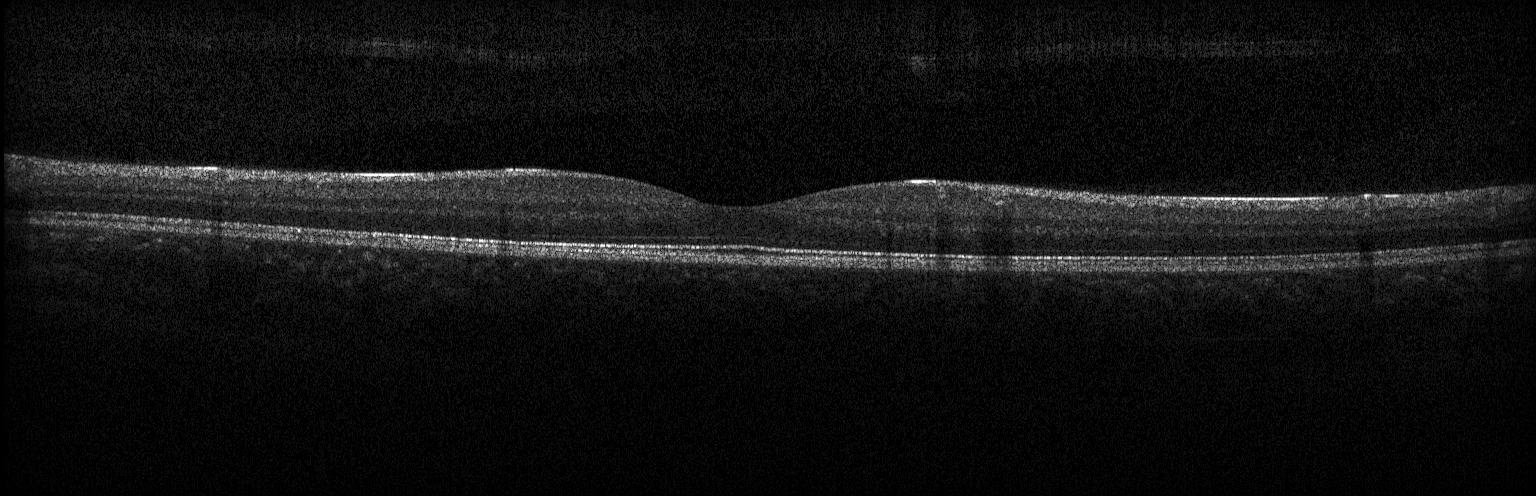

Optical coherence tomography B-scan. Macular scan. Heidelberg Spectralis OCT system.
Assessment: neither CNV, DME, nor drusen.